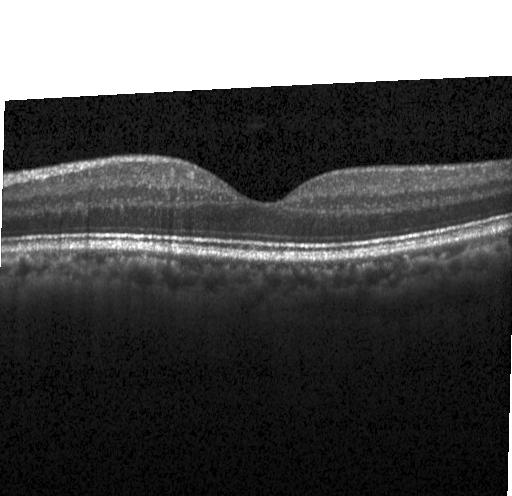
Retinal OCT cross-section
Diagnosis: no choroidal neovascularization, diabetic macular edema, or drusen.